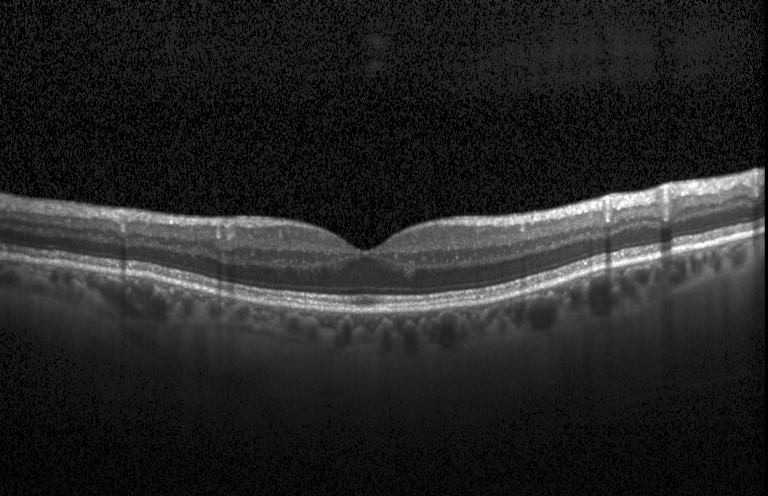

Retinal OCT cross-section · centered on the fovea · spectral-domain OCT — Assessment: no evidence of CNV, DME, or drusen.